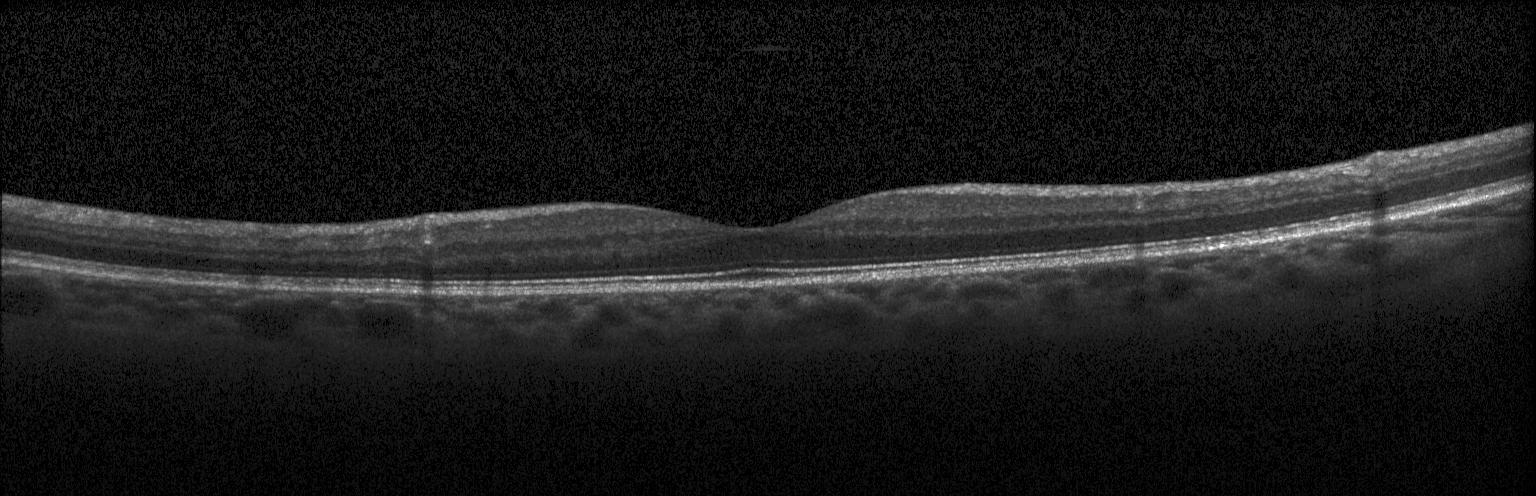 OCT finding: no evidence of CNV, DME, or drusen.